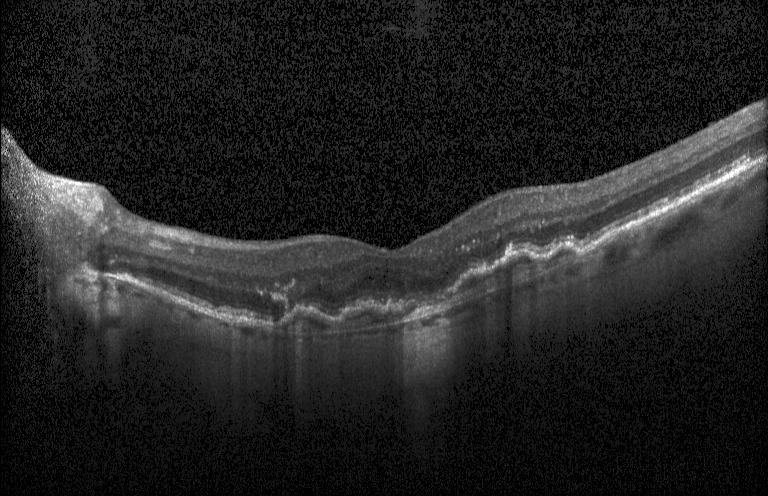 Retinal OCT cross-section; through the macula; Heidelberg Spectralis OCT system
The scan shows choroidal neovascularization (CNV).